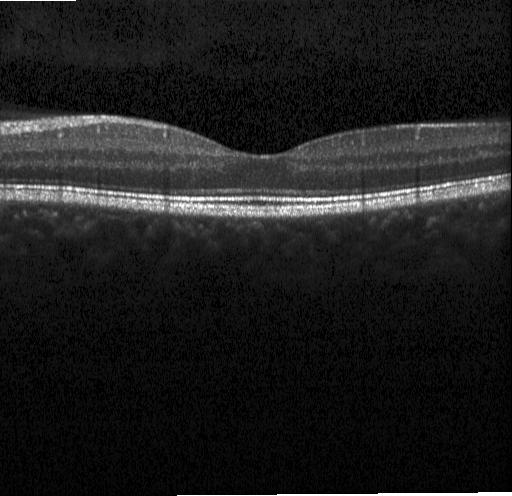

Diagnosis: no choroidal neovascularization, no diabetic macular edema, and no drusen.